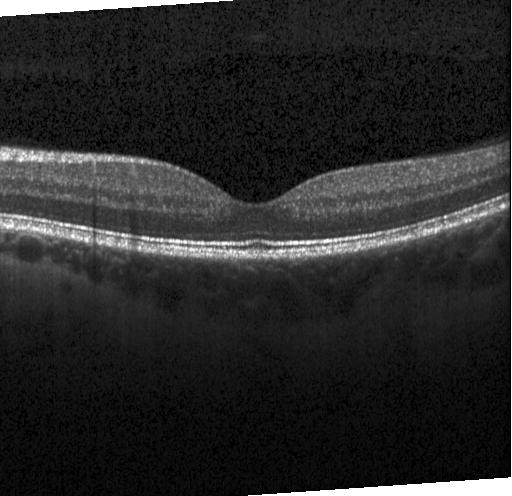
OCT line scan
The scan shows no CNV, no DME, and no drusen.